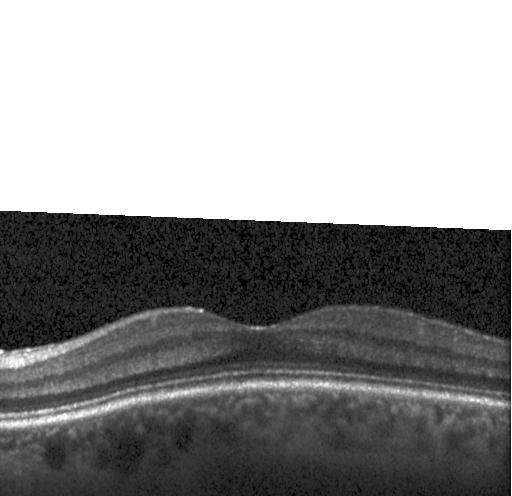 Fovea-centered, retinal OCT B-scan, spectral-domain OCT — Impression: no evidence of choroidal neovascularization, diabetic macular edema, or drusen.